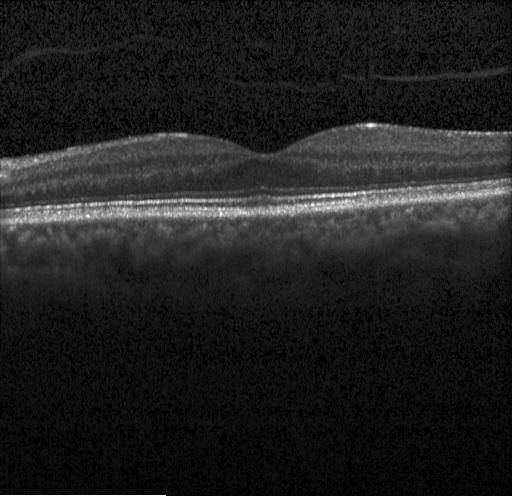

Centered on the fovea. Retinal OCT cross-section.
Diagnosis: neither choroidal neovascularization, diabetic macular edema, nor drusen.